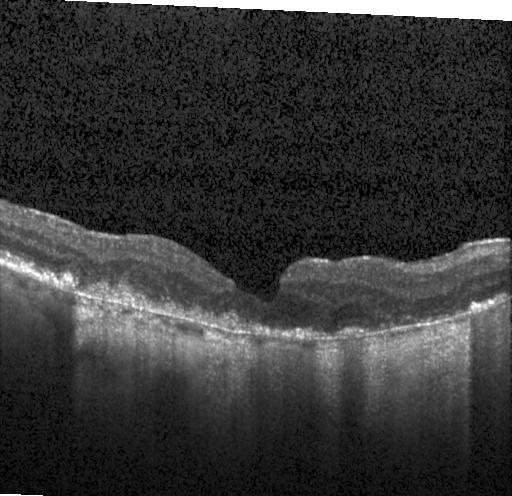
OCT B-scan, spectral-domain optical coherence tomography. Impression: a choroidal neovascular membrane.